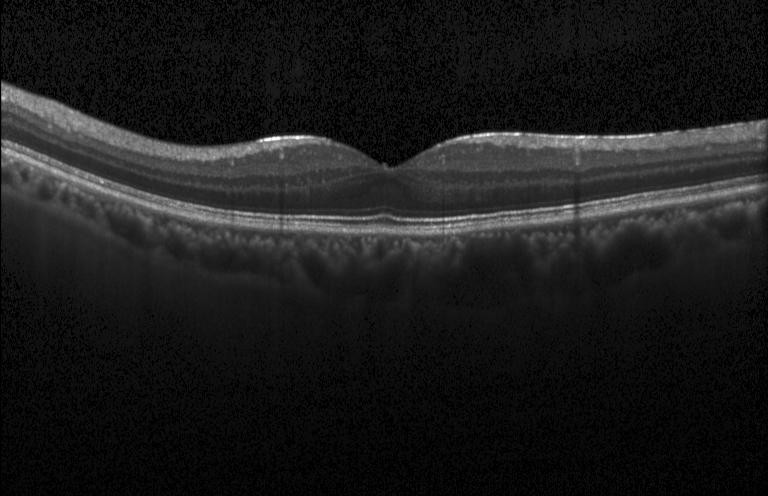

Macular OCT: no choroidal neovascularization, no diabetic macular edema, and no drusen.